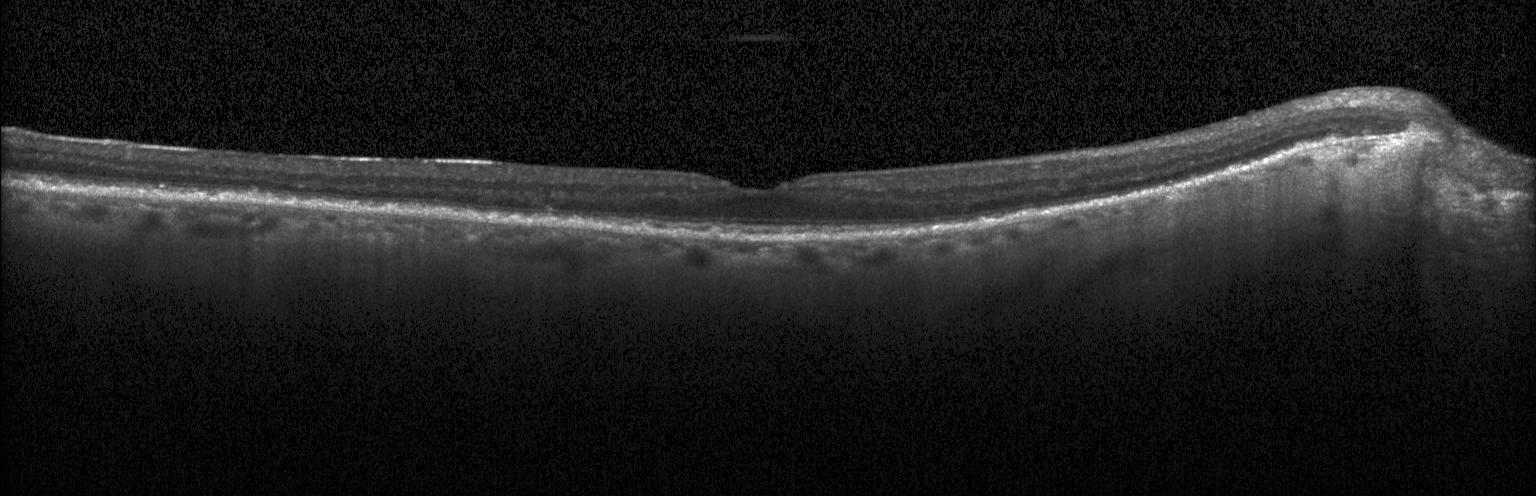

Optical coherence tomography scan — Macular OCT: drusen.